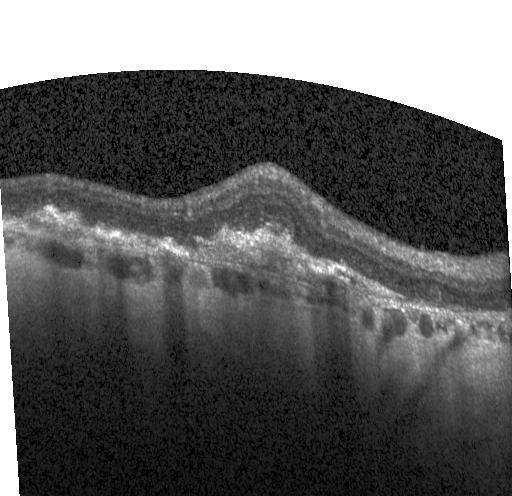
OCT B-scan
Finding: CNV.